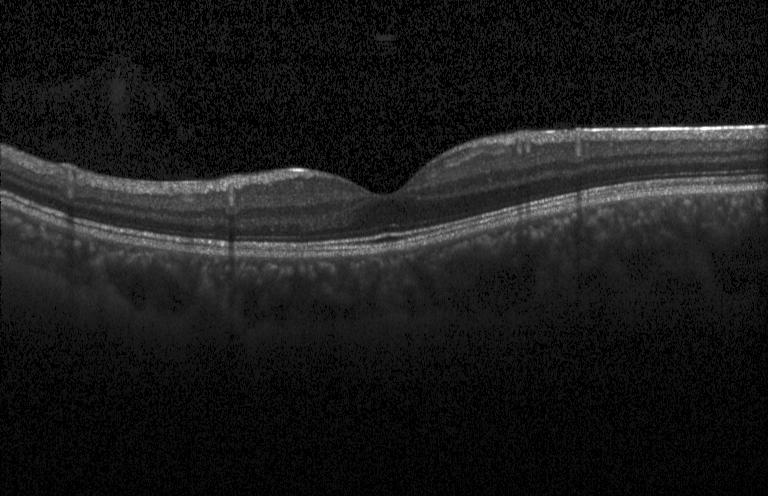

Spectral-domain OCT, OCT B-scan, acquired on a Heidelberg Spectralis
Dx: neither choroidal neovascularization, diabetic macular edema, nor drusen.